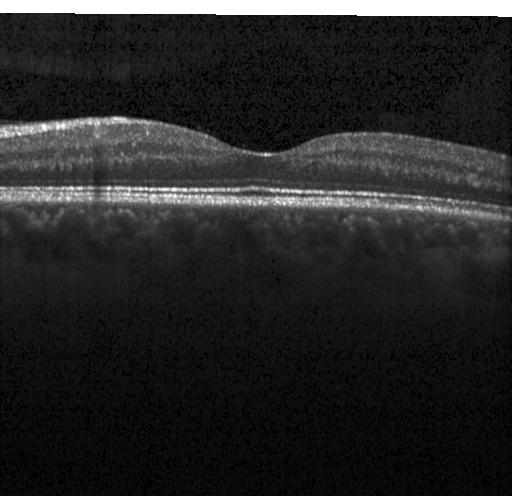
Finding: neither choroidal neovascularization, diabetic macular edema, nor drusen.